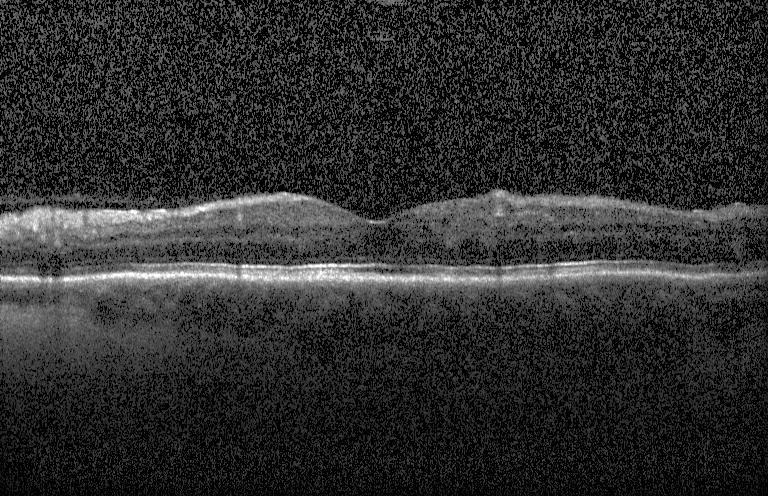

Retinal OCT B-scan · Heidelberg Spectralis · SD-OCT — Finding: diabetic macular edema (DME).